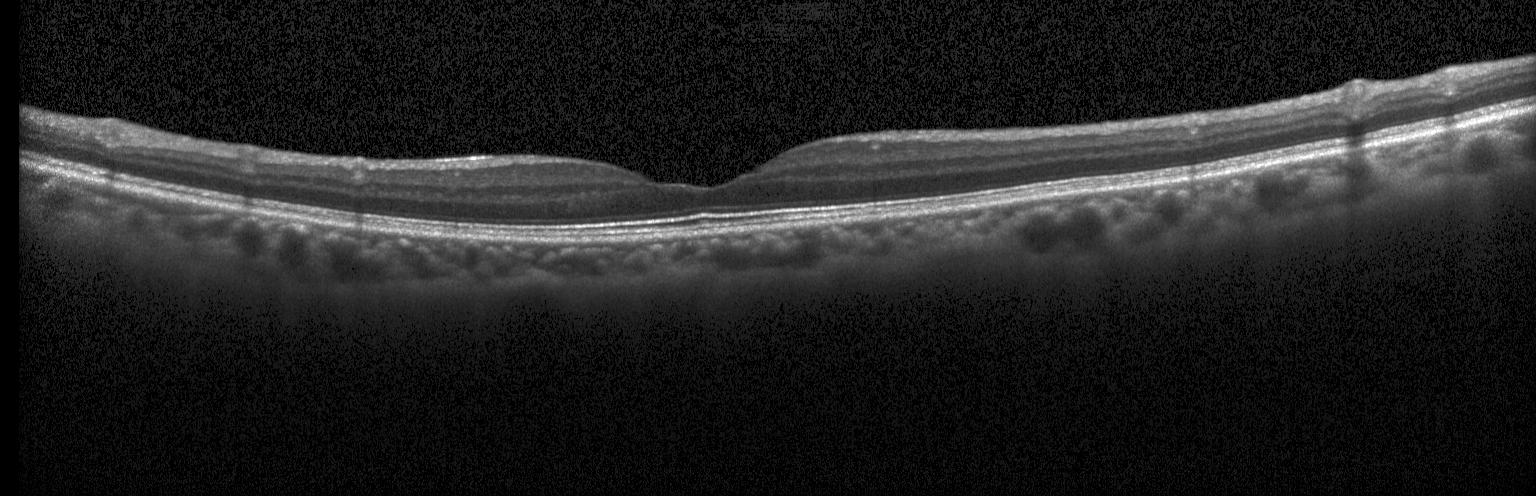 Diagnosis: no evidence of CNV, DME, or drusen.